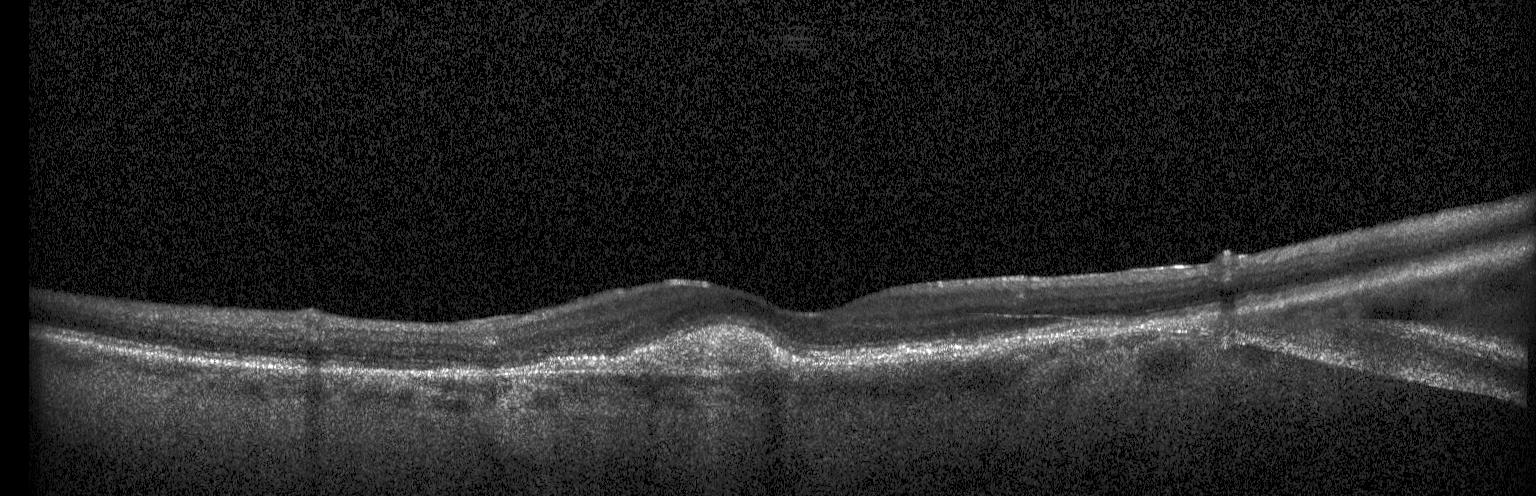

Spectral-domain optical coherence tomography, instrument: Heidelberg Spectralis, centered on the fovea, OCT line scan. Impression: choroidal neovascularization.